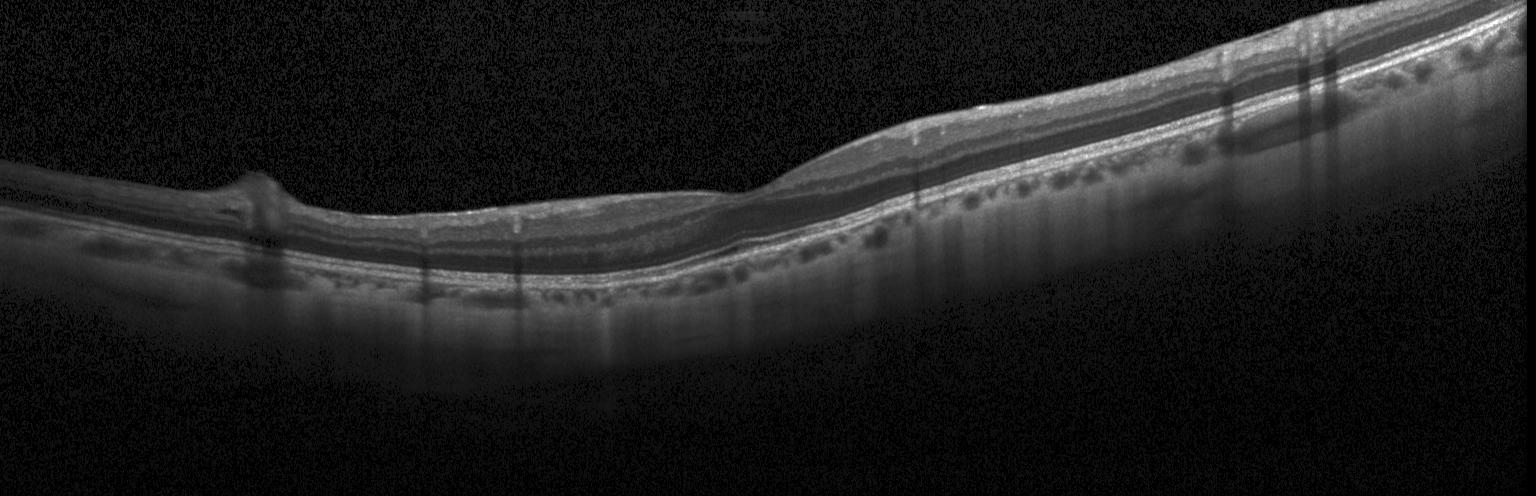

Macular scan. SD-OCT. Optical coherence tomography scan.
Assessment: no CNV, DME, or drusen.